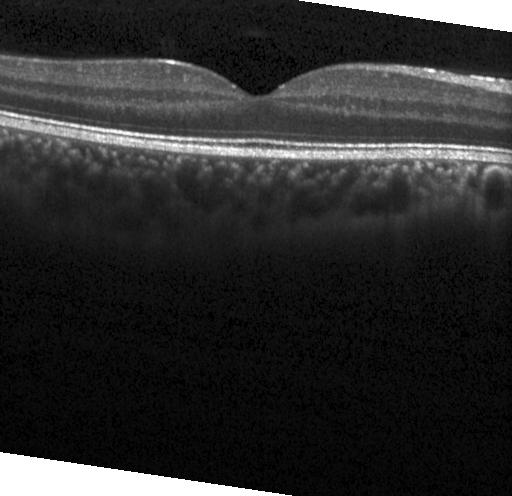
Heidelberg Spectralis OCT system; optical coherence tomography scan; through the macula. Dx: no choroidal neovascularization, no diabetic macular edema, and no drusen.